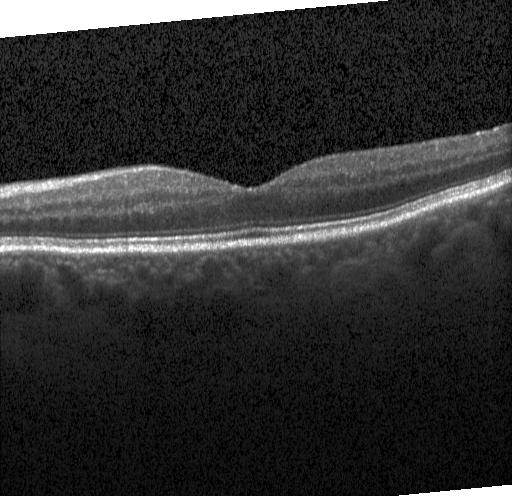 Instrument: Heidelberg Spectralis · OCT line scan · macular scan · SD-OCT. Macular OCT: no choroidal neovascularization, no diabetic macular edema, and no drusen.